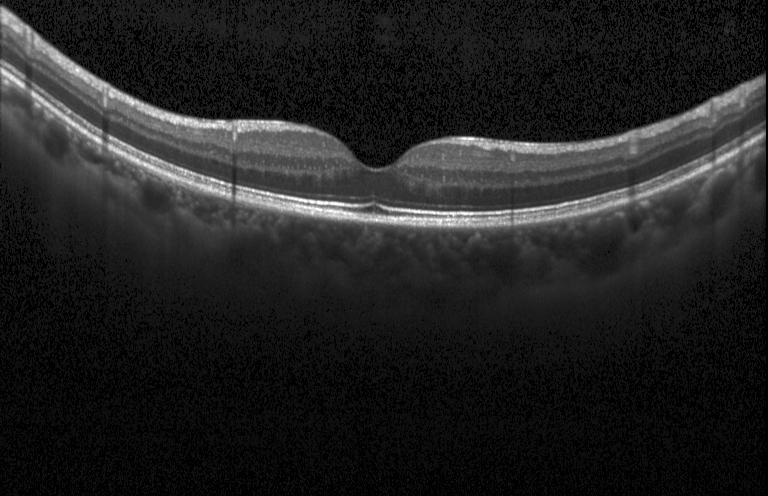 Optical coherence tomography B-scan
Diagnosis: neither CNV, DME, nor drusen.